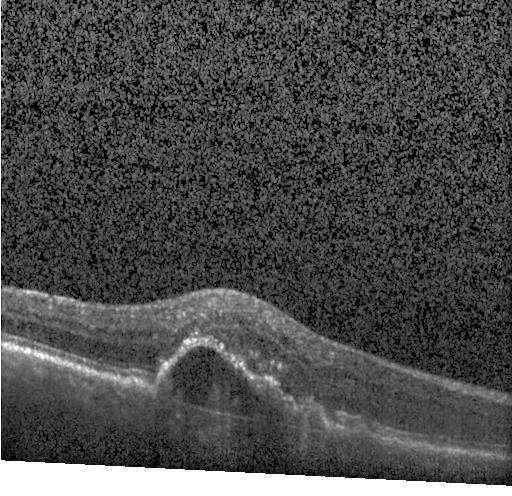 Retinal OCT B-scan, fovea-centered — Macular OCT: choroidal neovascularization.